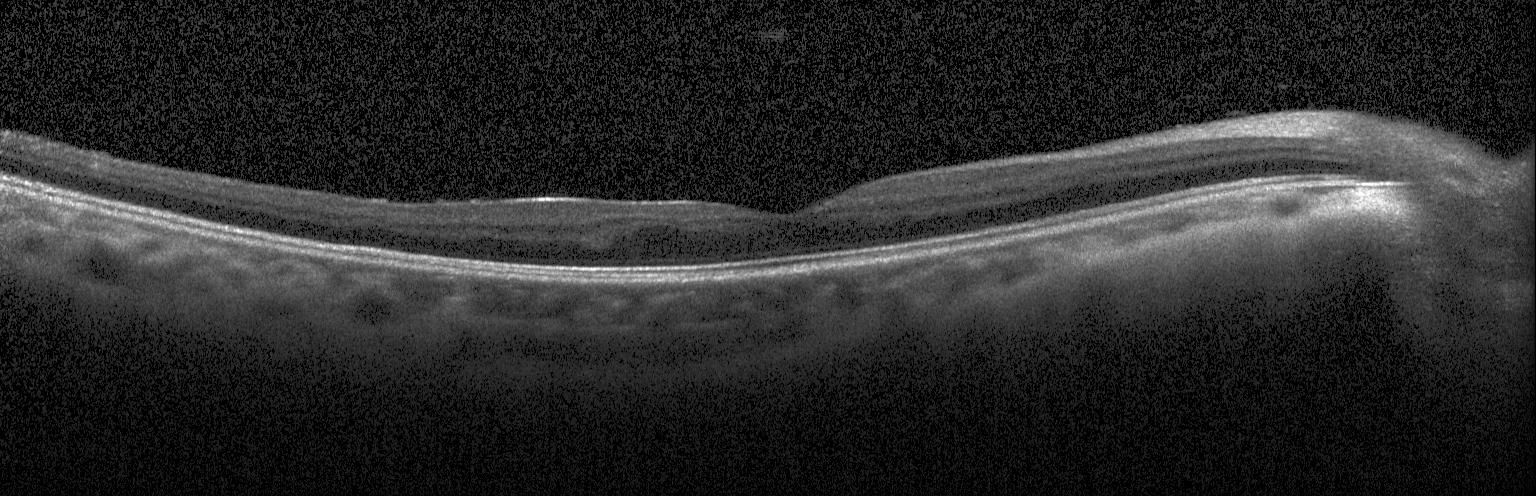 OCT line scan.
Macular OCT: no CNV, DME, or drusen.